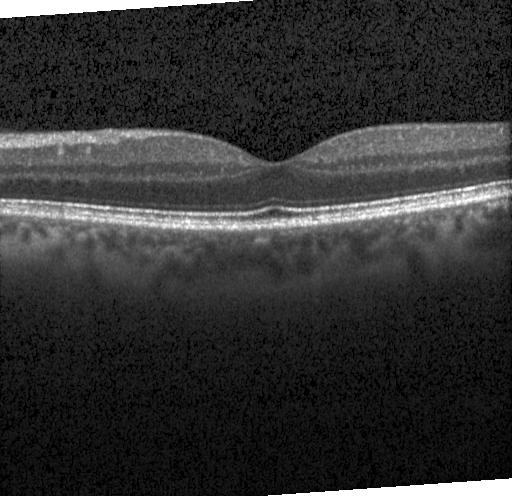
Finding: neither choroidal neovascularization, diabetic macular edema, nor drusen.